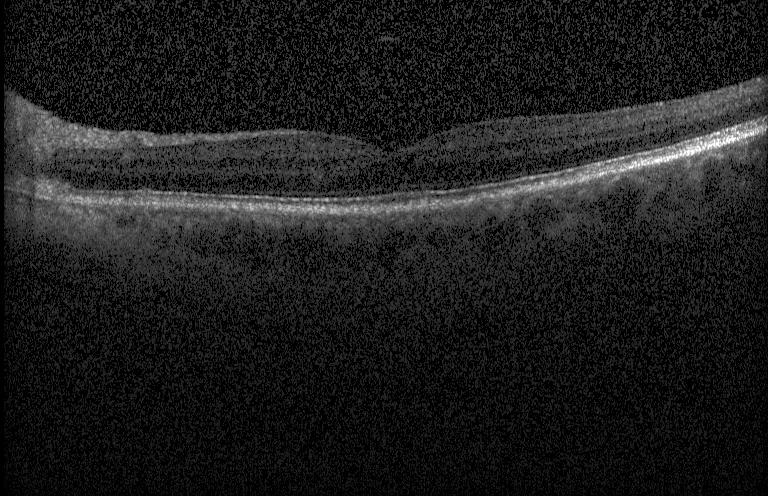

Retinal OCT cross-section. Finding: no evidence of choroidal neovascularization, diabetic macular edema, or drusen.